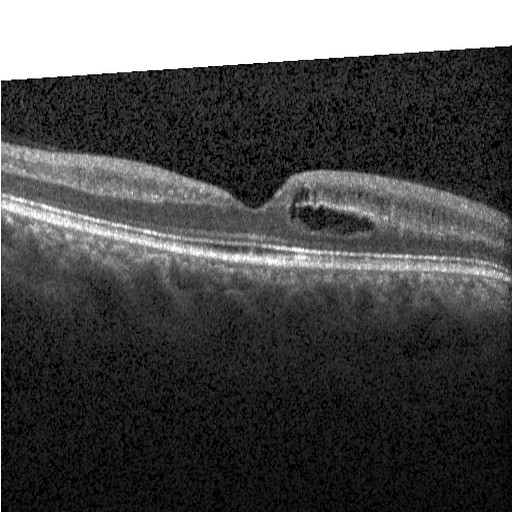

Retinal OCT B-scan — Diagnosis: diabetic macular edema.